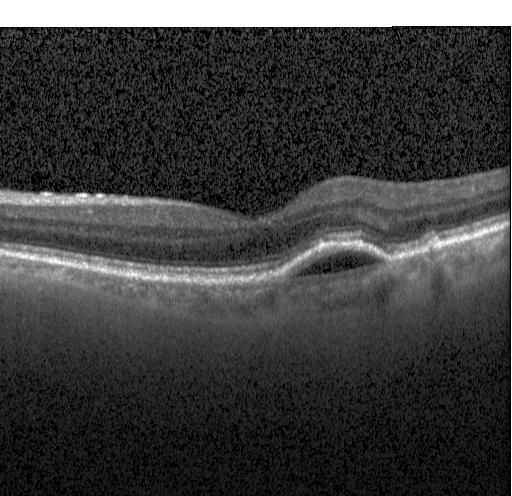 Optical coherence tomography B-scan.
Assessment: a choroidal neovascular membrane.